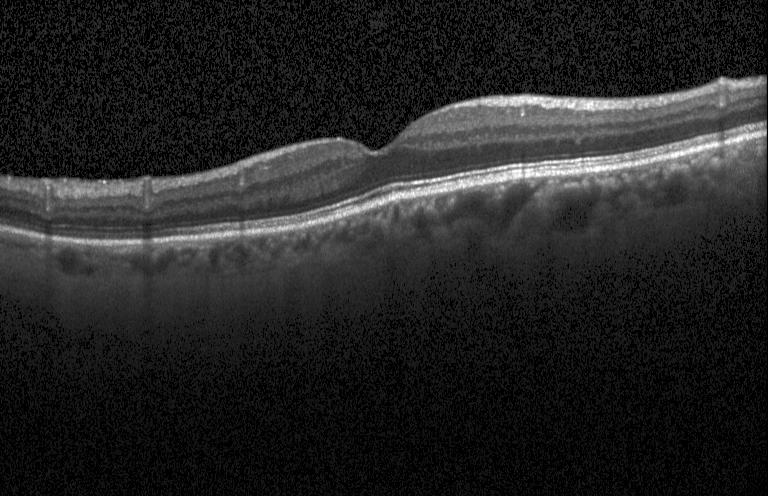
OCT line scan; acquired on a Heidelberg Spectralis; through the macula. OCT finding: no evidence of CNV, DME, or drusen.